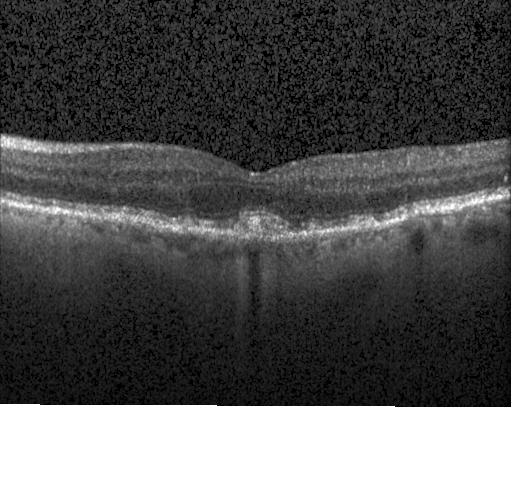

Macular OCT: drusen.